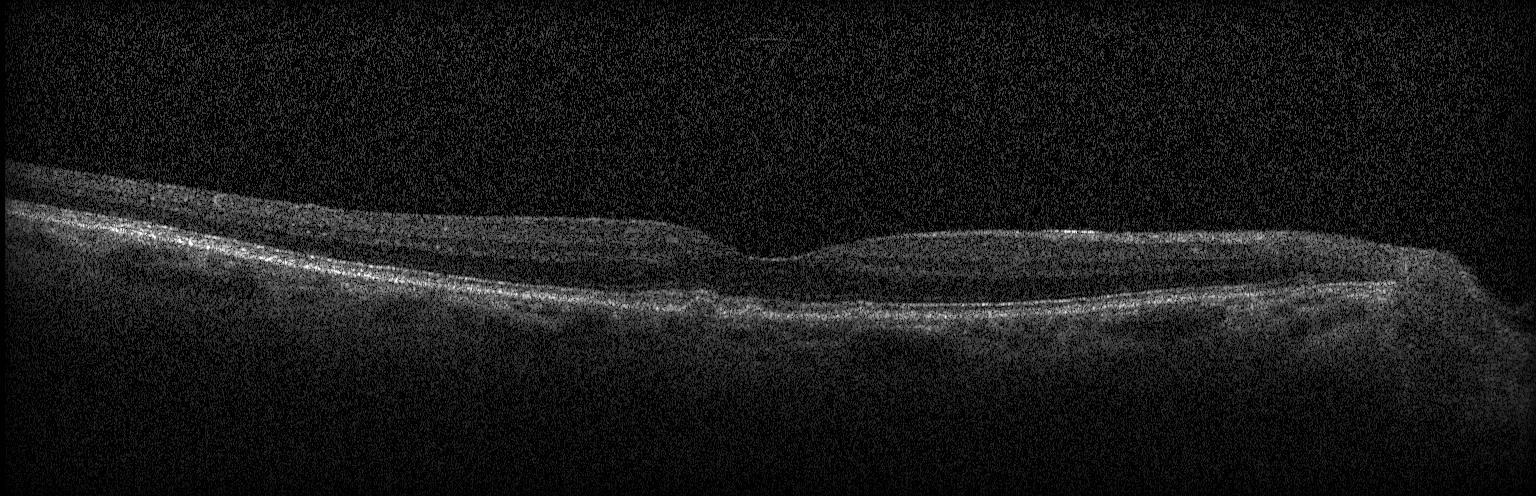 Retinal OCT cross-section showing multiple drusen.